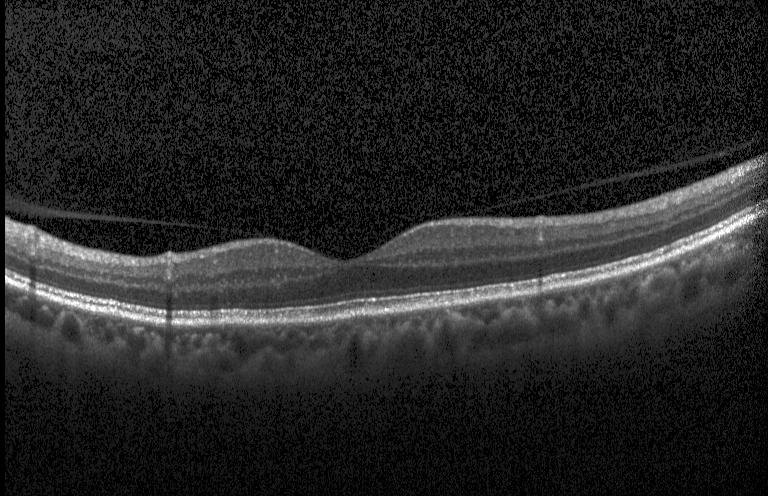

Spectral-domain OCT. Centered on the fovea. OCT line scan. Acquired on a Heidelberg Spectralis
Assessment: no CNV, DME, or drusen.